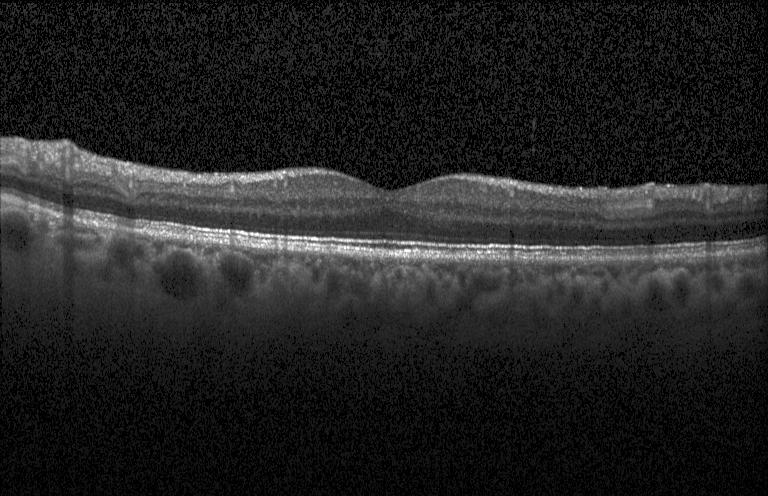
Retinal OCT B-scan
Macular OCT: no CNV, no DME, and no drusen.